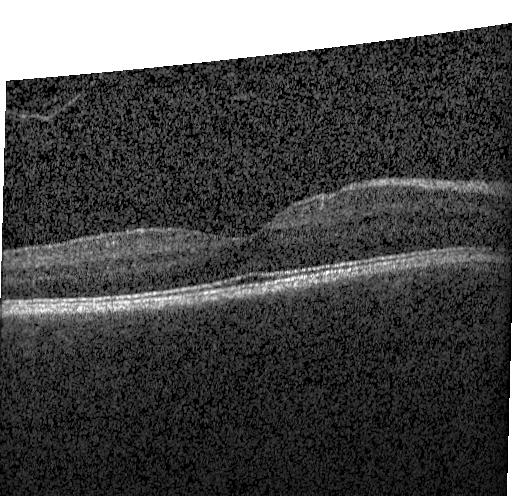 Finding: neither choroidal neovascularization, diabetic macular edema, nor drusen.